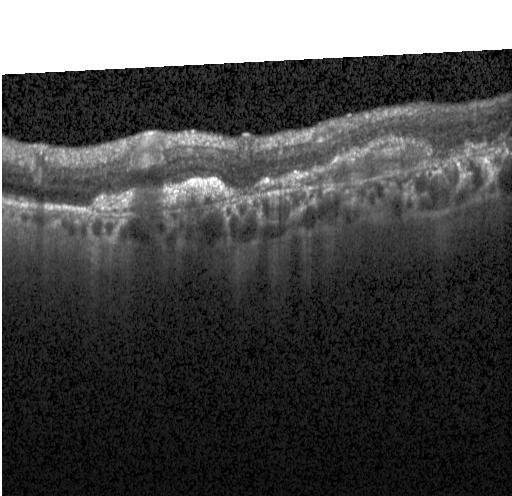 Heidelberg Spectralis OCT system, OCT line scan
Impression: choroidal neovascularization.